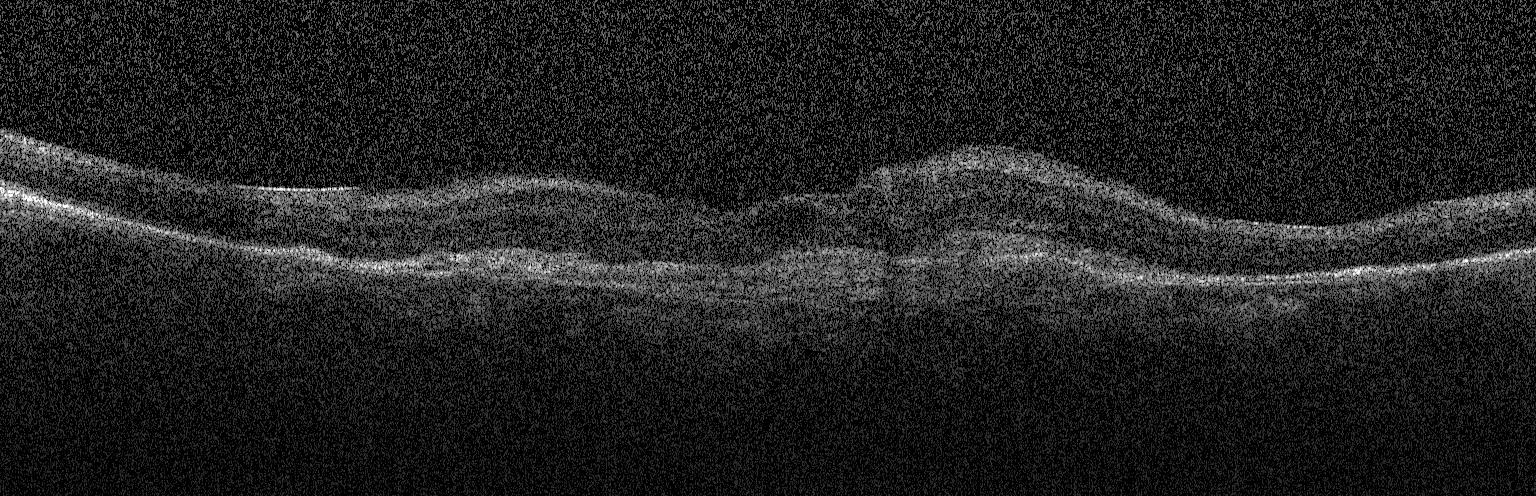

Finding: choroidal neovascularization.